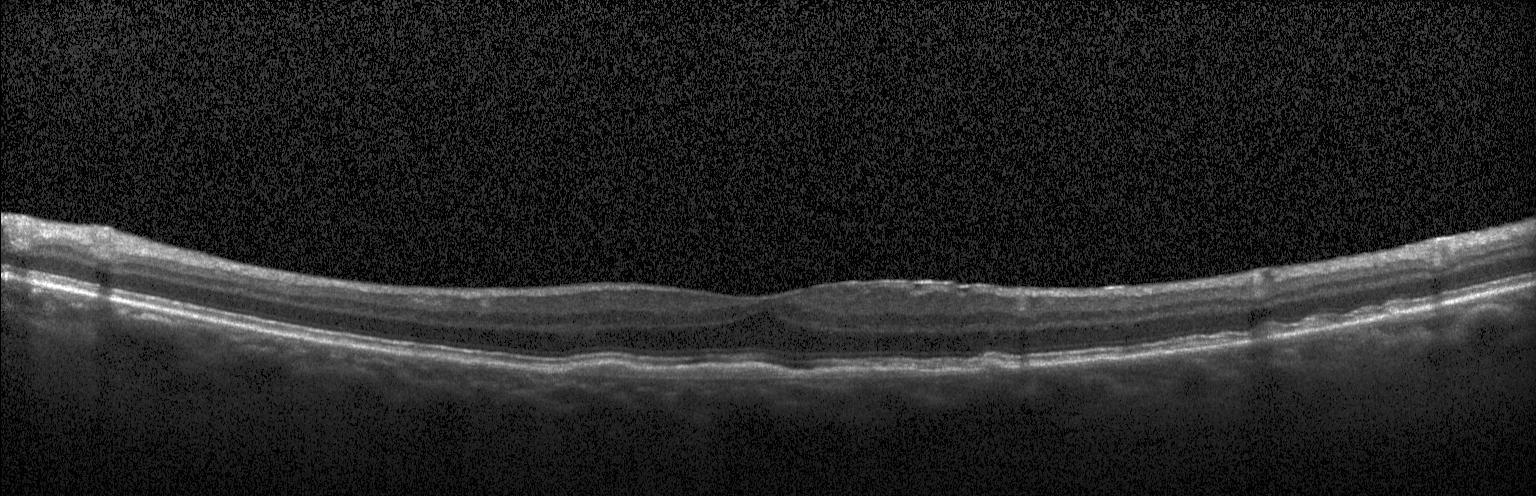

This B-scan demonstrates a choroidal neovascular membrane.